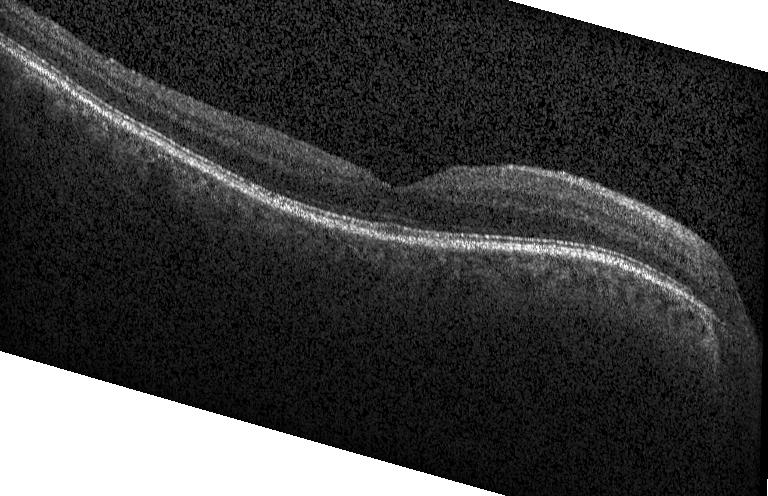
Impression: no evidence of choroidal neovascularization, diabetic macular edema, or drusen.